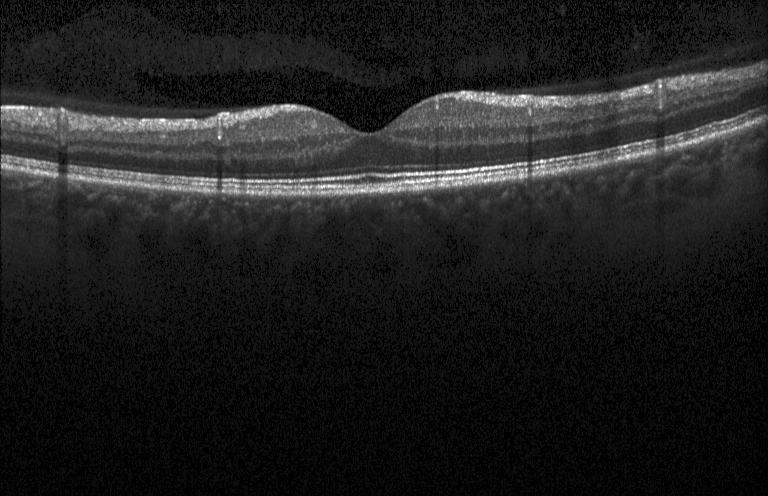
Retinal OCT cross-section, through the macula — Impression: no CNV, no DME, and no drusen.